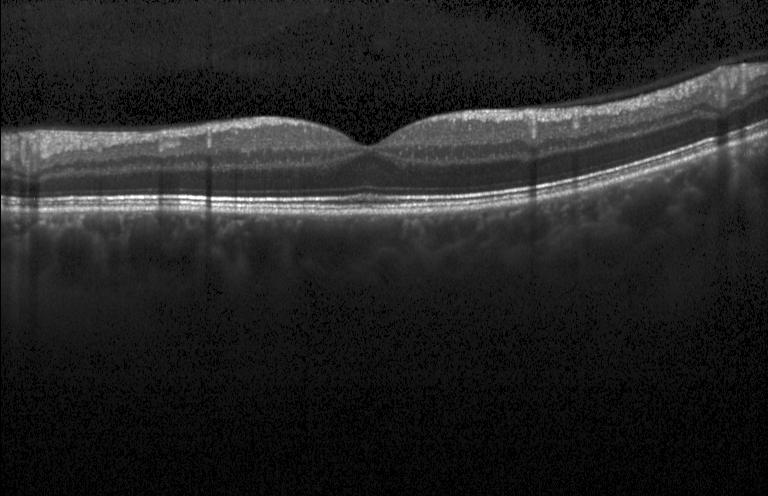

OCT line scan; instrument: Heidelberg Spectralis.
This B-scan demonstrates neither choroidal neovascularization, diabetic macular edema, nor drusen.